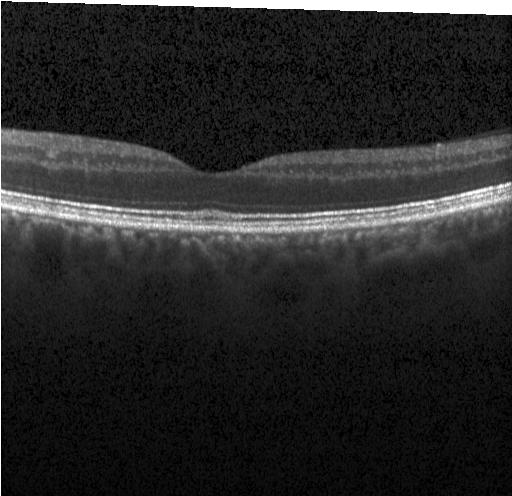 Retinal OCT B-scan. Centered on the fovea. Instrument: Heidelberg Spectralis. Spectral-domain optical coherence tomography — The scan shows no choroidal neovascularization, diabetic macular edema, or drusen.